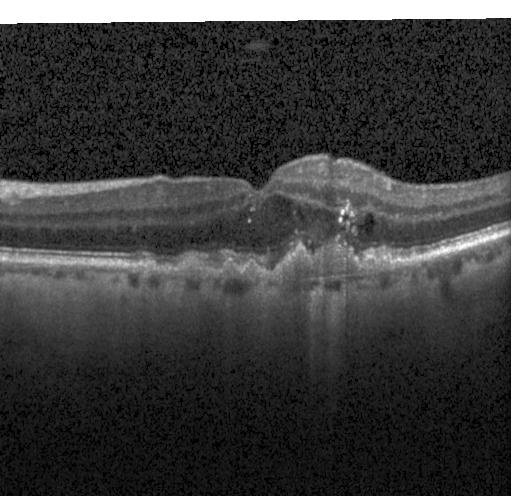
Dx: a choroidal neovascular membrane.